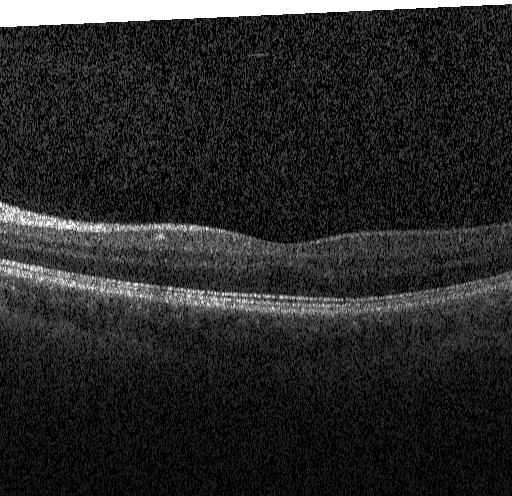 Optical coherence tomography scan. Heidelberg Spectralis. Impression: no evidence of choroidal neovascularization, diabetic macular edema, or drusen.